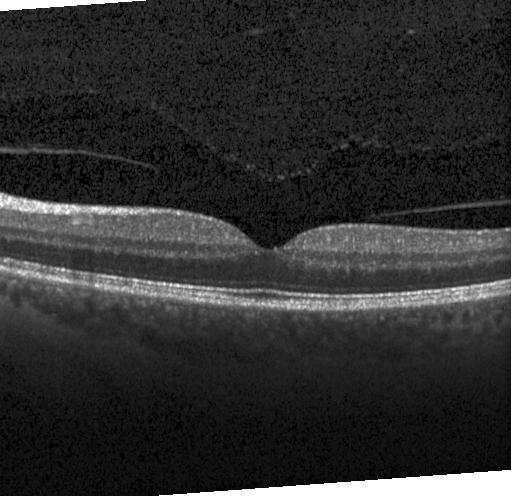 Retinal OCT B-scan · centered on the fovea · Heidelberg Spectralis OCT system.
OCT finding: no CNV, DME, or drusen.